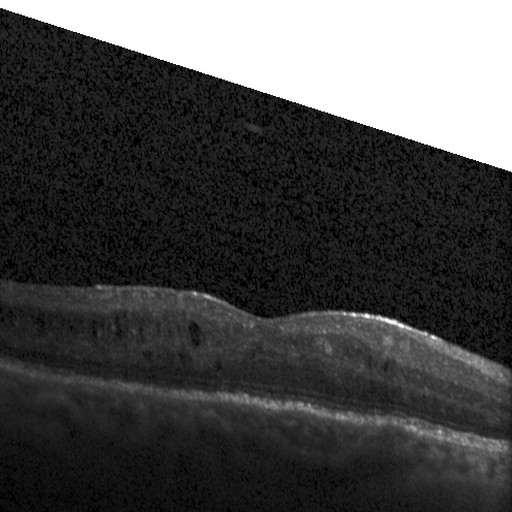
Spectral-domain OCT B-scan: DME.